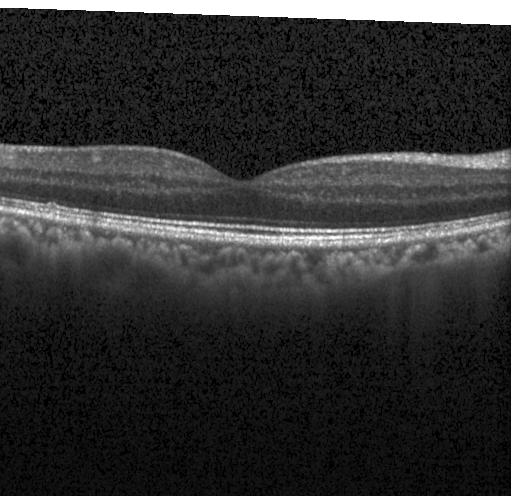

Through the macula. Retinal OCT B-scan — Dx: no evidence of CNV, DME, or drusen.